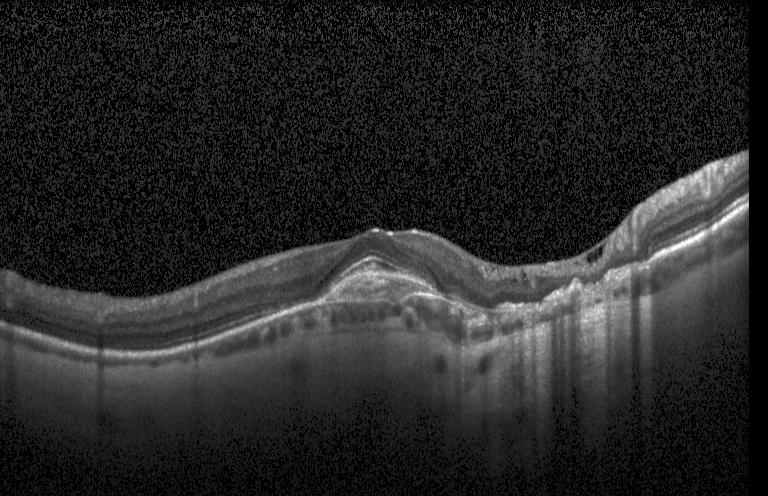 Heidelberg Spectralis · optical coherence tomography B-scan. This B-scan demonstrates a choroidal neovascular membrane.